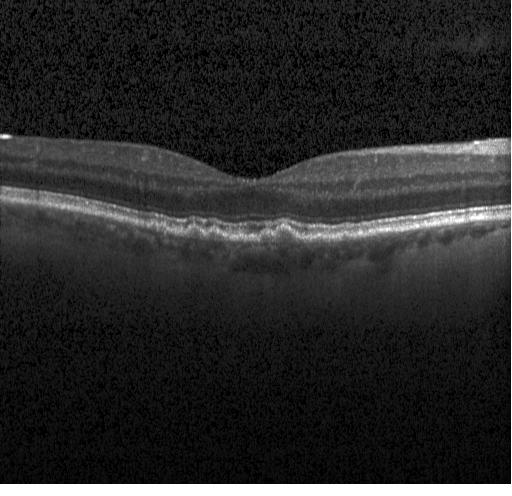 Through the macula · instrument: Heidelberg Spectralis · retinal OCT B-scan. This B-scan demonstrates drusen.